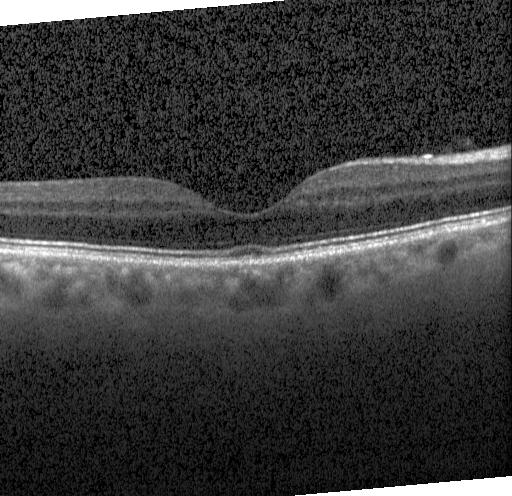

Diagnosis: no CNV, no DME, and no drusen.